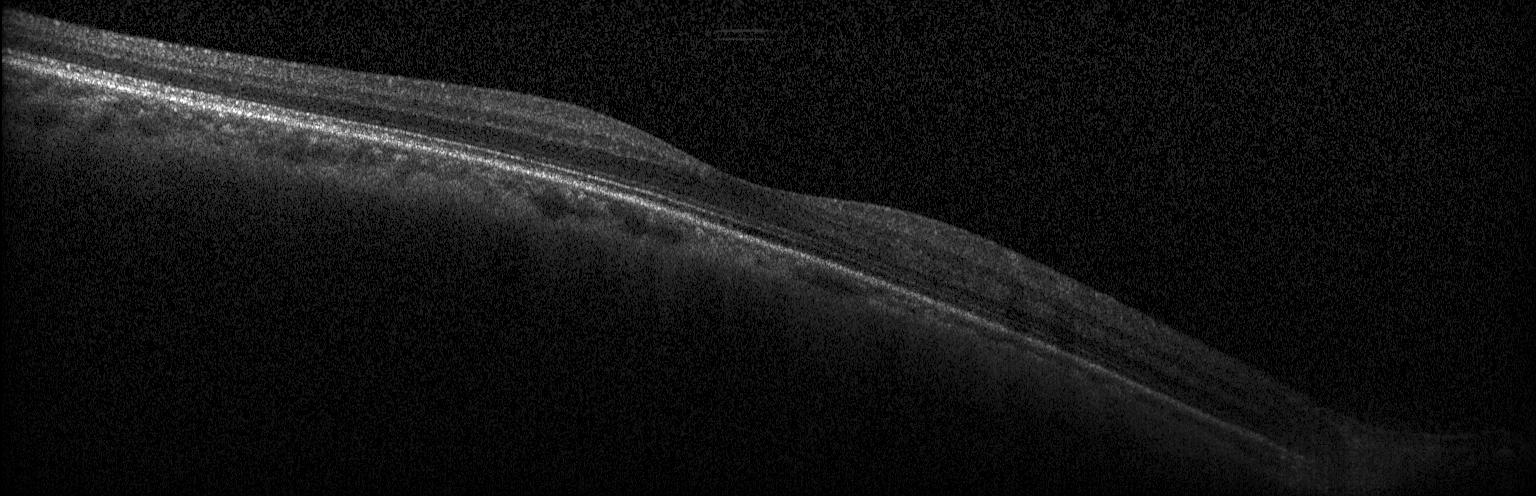

Neither choroidal neovascularization, diabetic macular edema, nor drusen.